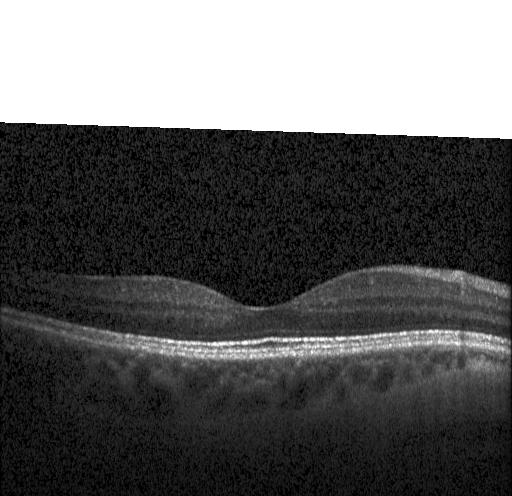 Diagnosis: neither CNV, DME, nor drusen.